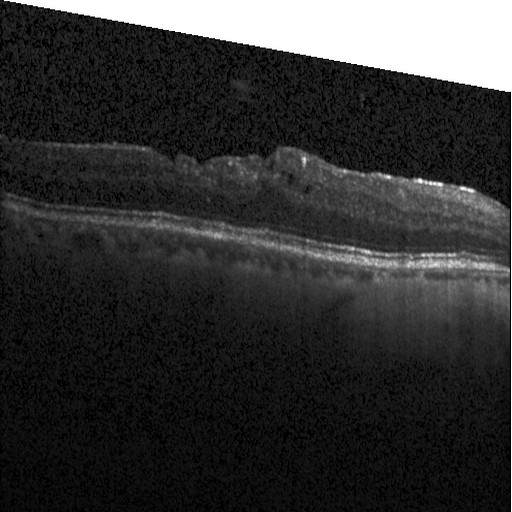

OCT line scan; through the macula
Finding: diabetic macular edema (DME).